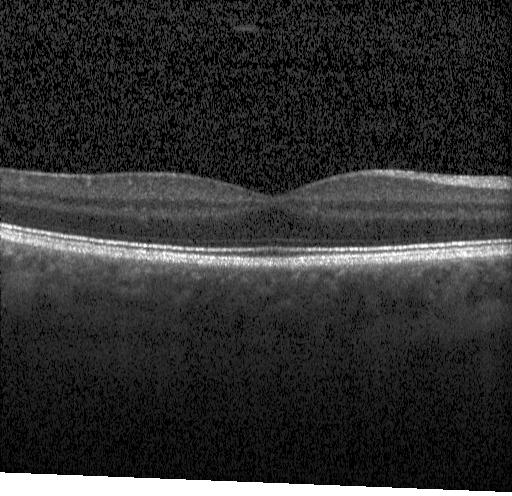

OCT line scan; acquired on a Heidelberg Spectralis
Finding: neither choroidal neovascularization, diabetic macular edema, nor drusen.